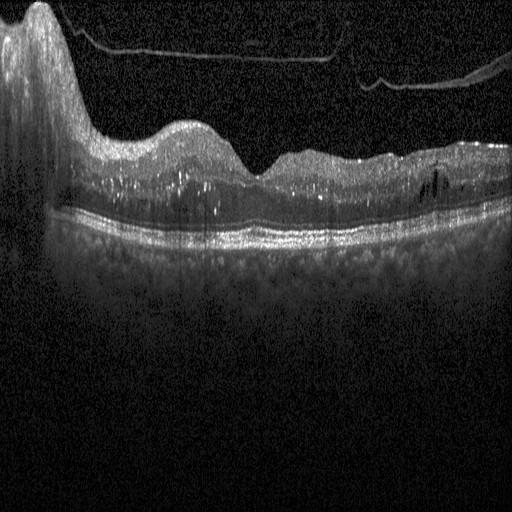
Assessment: diabetic macular edema.